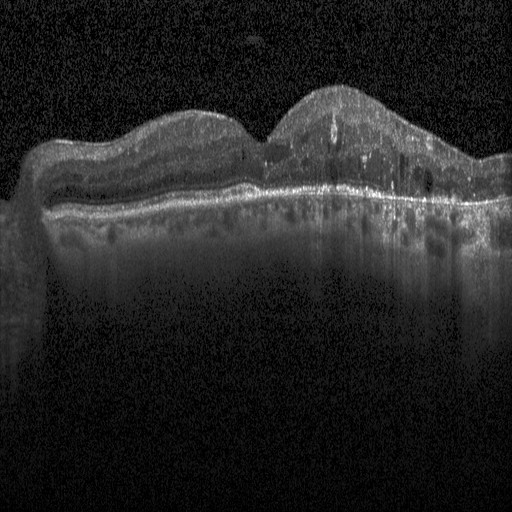

Impression: diabetic macular edema.